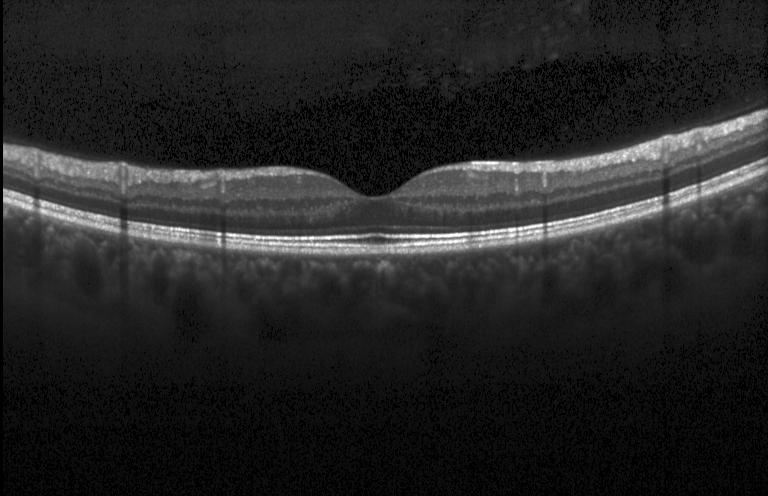
Finding: no choroidal neovascularization, no diabetic macular edema, and no drusen.